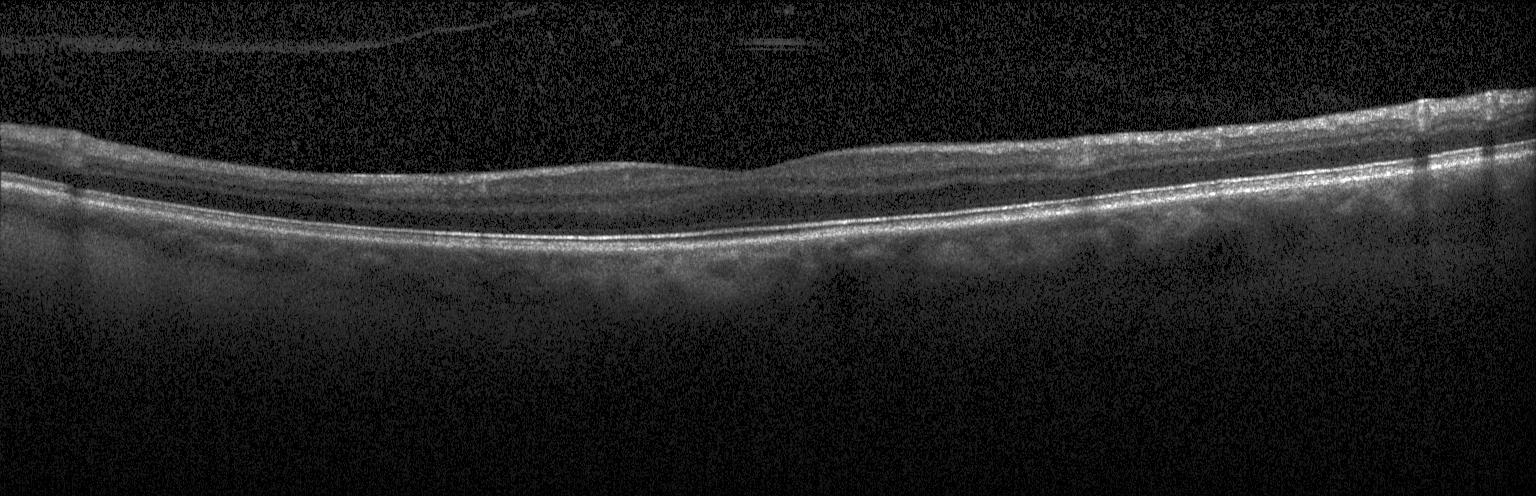
SD-OCT; optical coherence tomography B-scan — Diagnosis: neither choroidal neovascularization, diabetic macular edema, nor drusen.